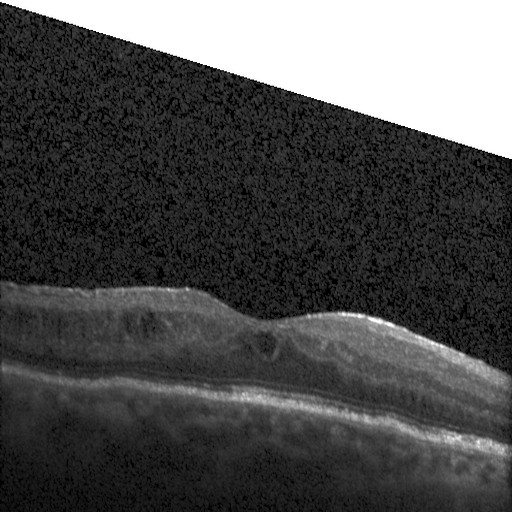 Heidelberg Spectralis OCT system. Retinal OCT cross-section. OCT finding: DME.